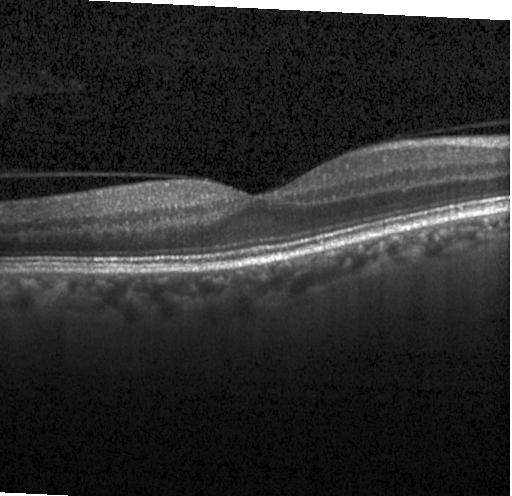

Retinal OCT B-scan
Impression: no evidence of CNV, DME, or drusen.